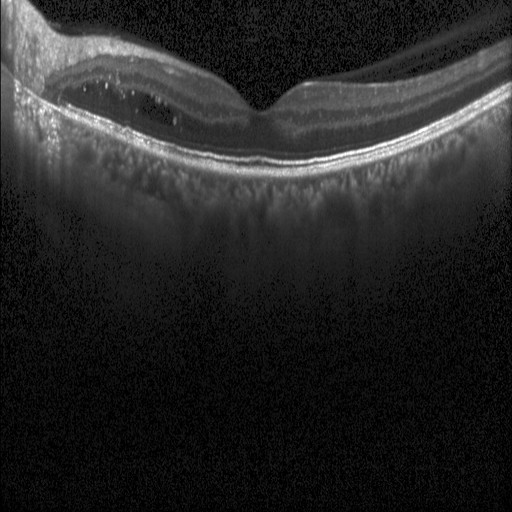

This B-scan demonstrates diabetic macular edema.